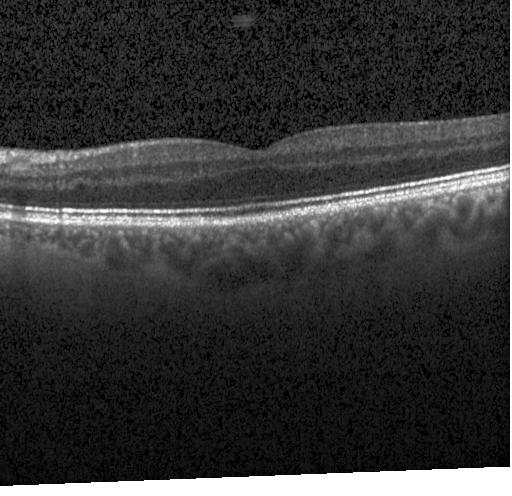 Macular OCT demonstrating no evidence of choroidal neovascularization, diabetic macular edema, or drusen.